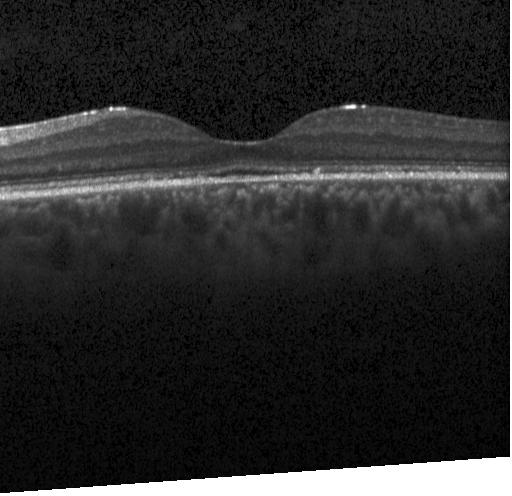
Optical coherence tomography B-scan
Finding: no CNV, no DME, and no drusen.